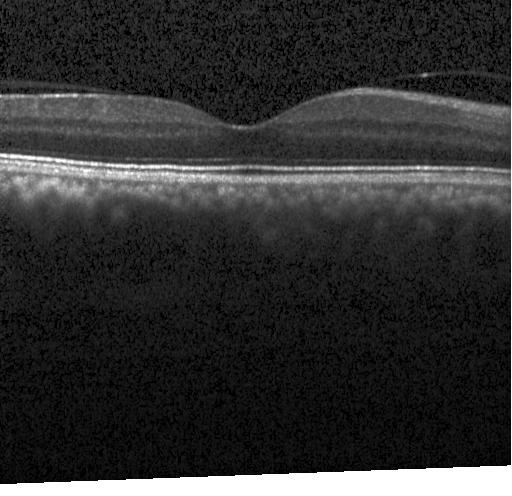
Horizontal scan through the fovea · optical coherence tomography B-scan · Heidelberg Spectralis OCT system. Macular OCT: neither choroidal neovascularization, diabetic macular edema, nor drusen.